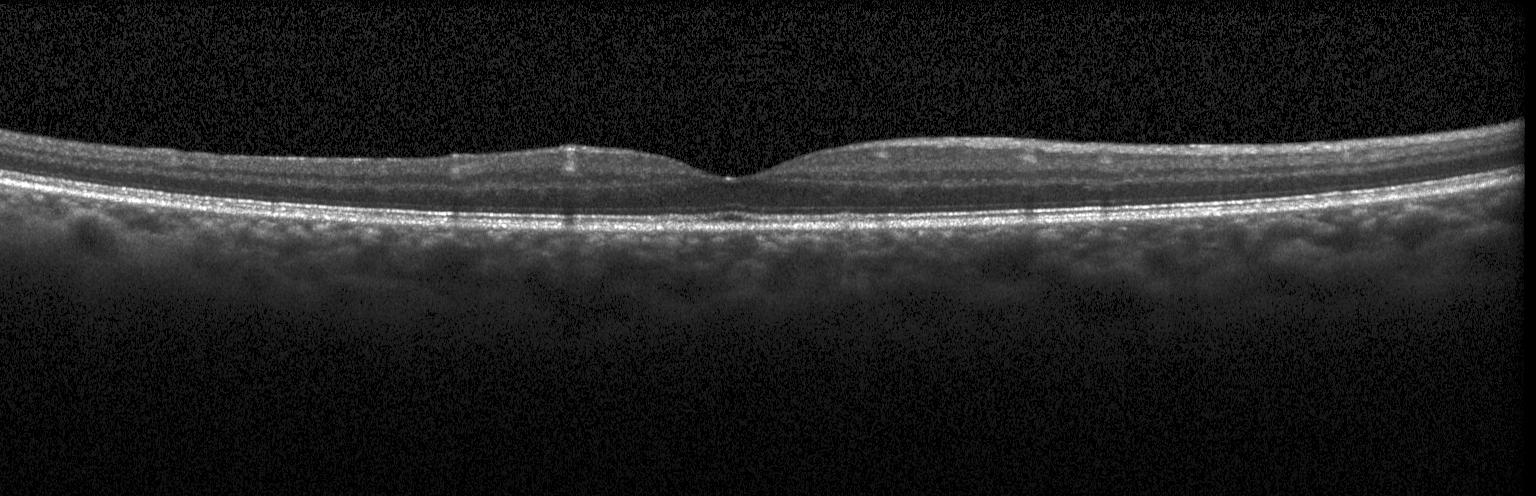
Optical coherence tomography B-scan — This B-scan demonstrates no evidence of choroidal neovascularization, diabetic macular edema, or drusen.